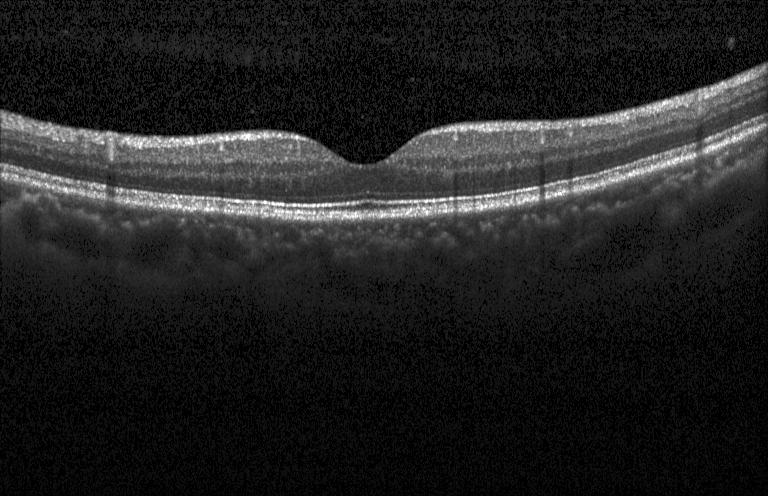 OCT line scan; instrument: Heidelberg Spectralis; through the macula. Finding: no choroidal neovascularization, diabetic macular edema, or drusen.